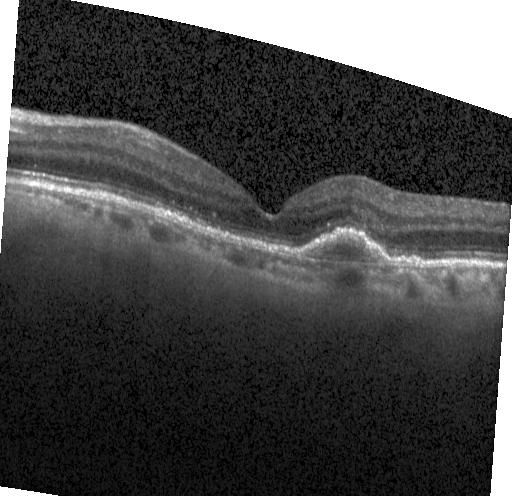

Diagnosis: choroidal neovascularization.